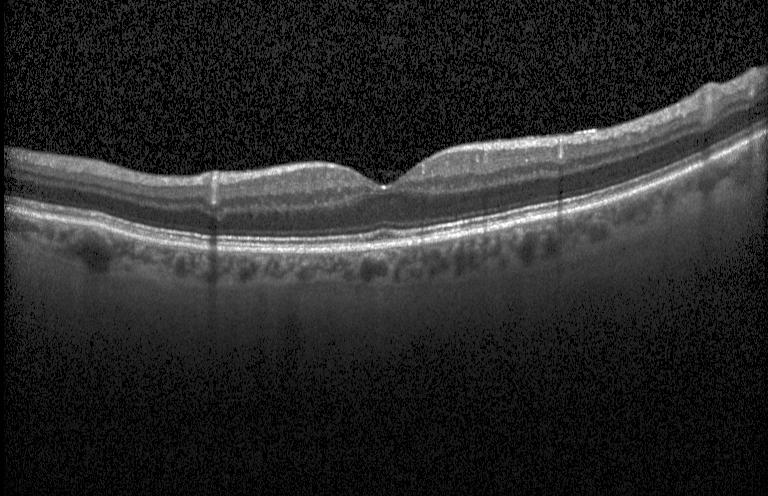 Assessment: no evidence of CNV, DME, or drusen.